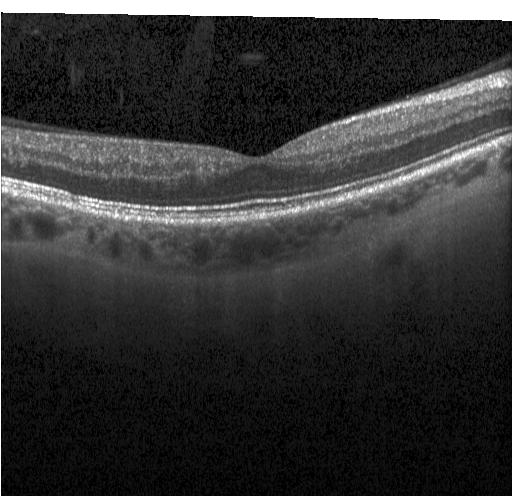
Optical coherence tomography B-scan. Through the macula. Dx: no choroidal neovascularization, diabetic macular edema, or drusen.